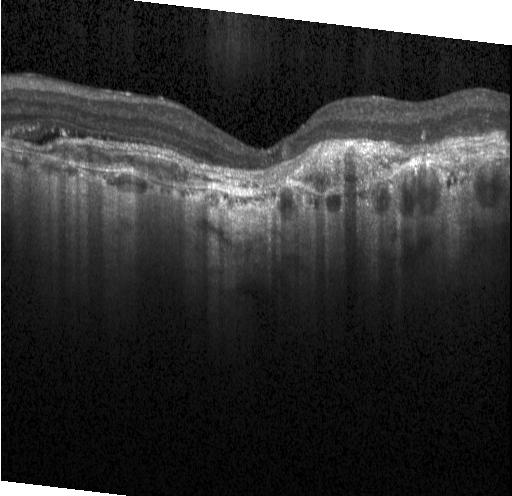

SD-OCT; fovea-centered; OCT line scan.
Impression: choroidal neovascularization (CNV).